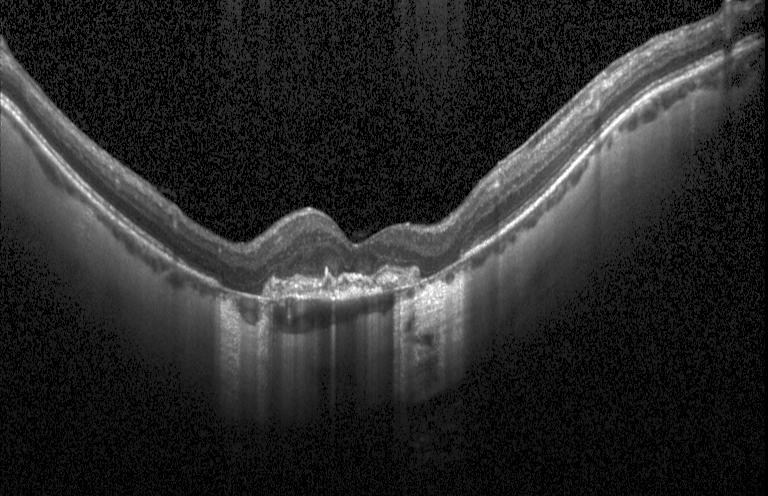

Optical coherence tomography B-scan
Finding: a choroidal neovascular membrane.